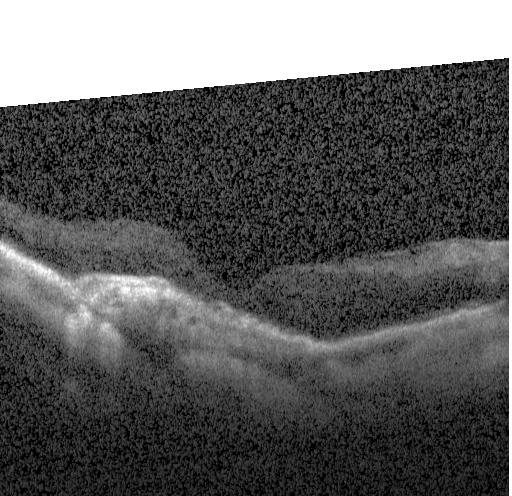

The scan shows a choroidal neovascular membrane.